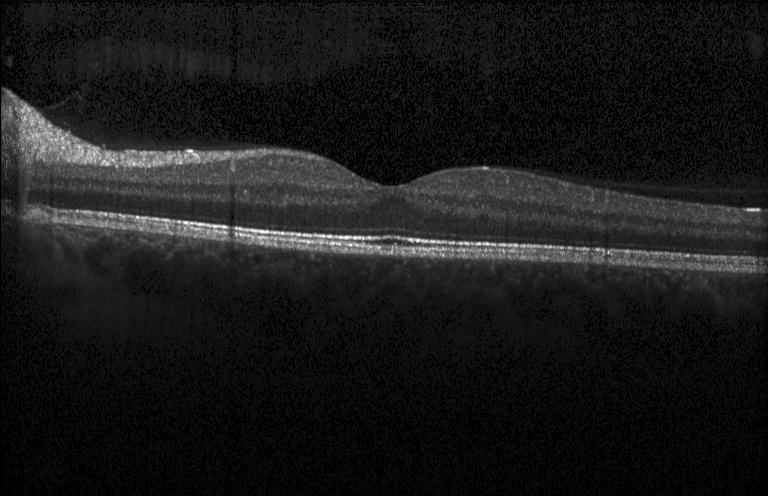 Spectral-domain OCT · retinal OCT B-scan
Dx: no CNV, no DME, and no drusen.